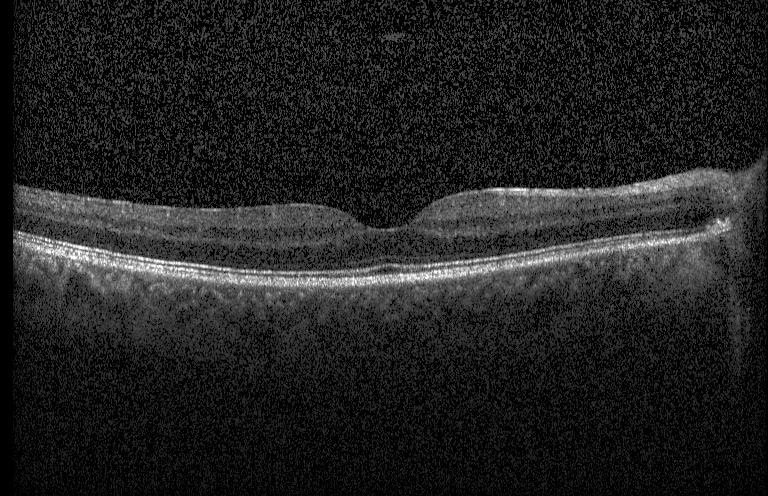
SD-OCT · instrument: Heidelberg Spectralis · optical coherence tomography B-scan · fovea-centered.
Dx: neither choroidal neovascularization, diabetic macular edema, nor drusen.